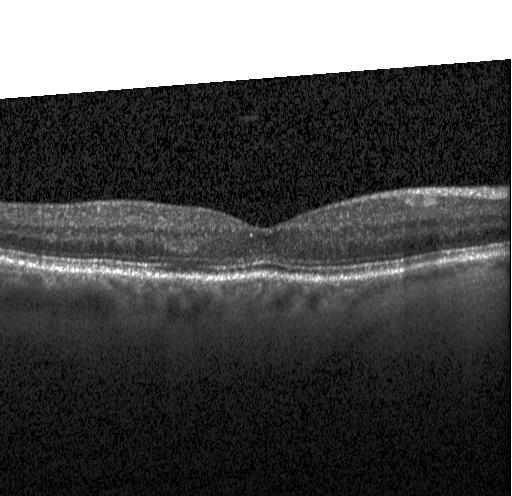 Retinal OCT B-scan — Diagnosis: neither choroidal neovascularization, diabetic macular edema, nor drusen.